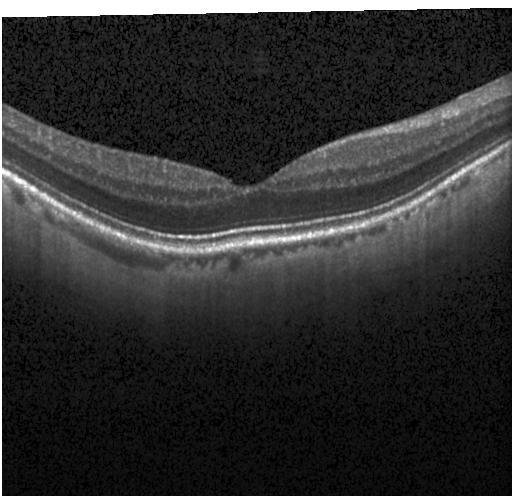

SD-OCT; optical coherence tomography B-scan; through the macula; acquired on a Heidelberg Spectralis.
Diagnosis: neither choroidal neovascularization, diabetic macular edema, nor drusen.